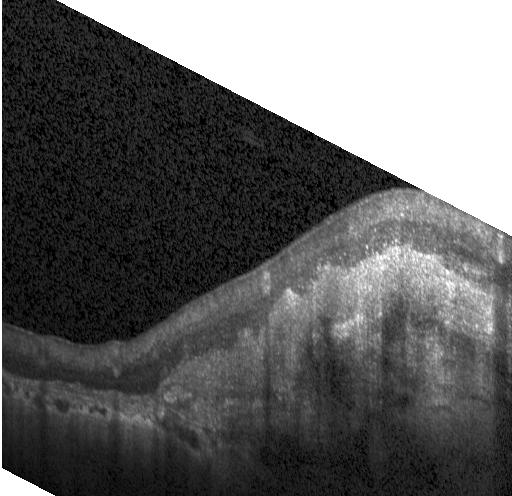 OCT B-scan · fovea-centered.
Impression: choroidal neovascularization.